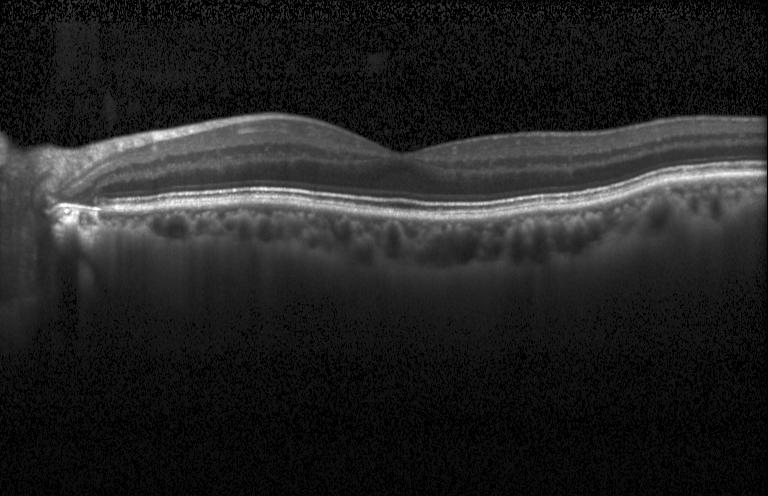
Retinal OCT B-scan
Finding: neither choroidal neovascularization, diabetic macular edema, nor drusen.